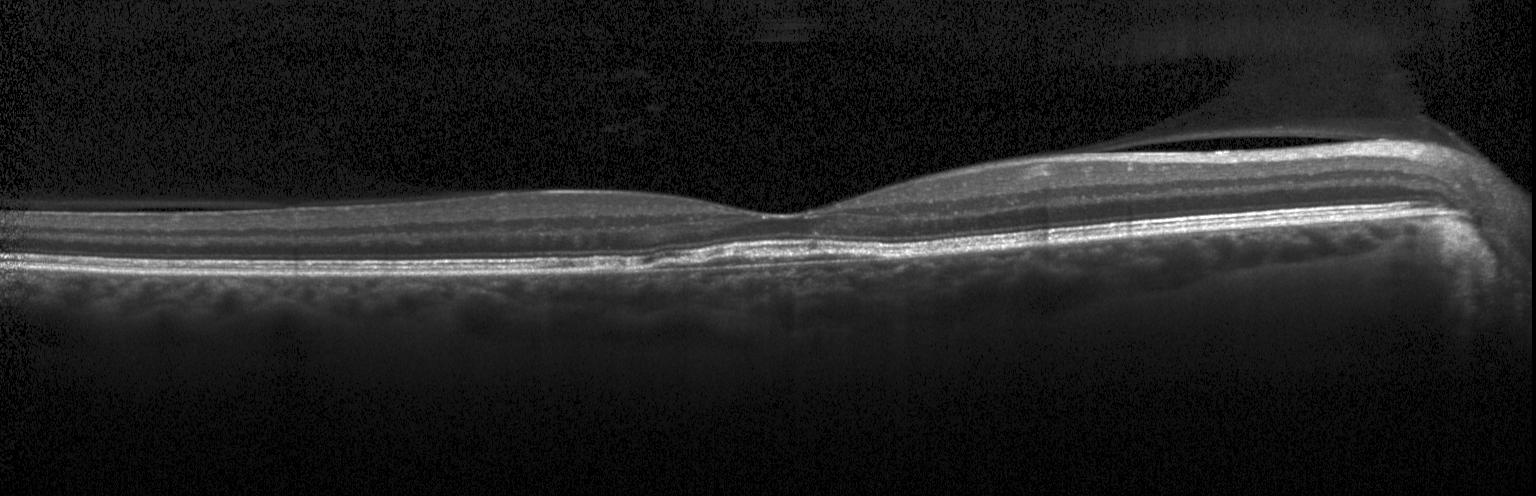
OCT line scan
Diagnosis: a choroidal neovascular membrane.